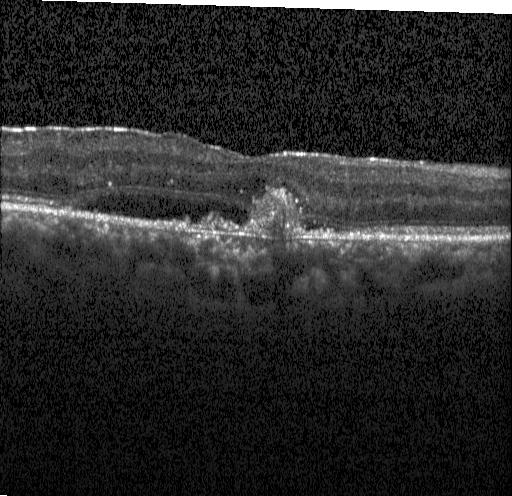

Optical coherence tomography scan. Instrument: Heidelberg Spectralis. Spectral-domain OCT — Dx: a choroidal neovascular membrane.